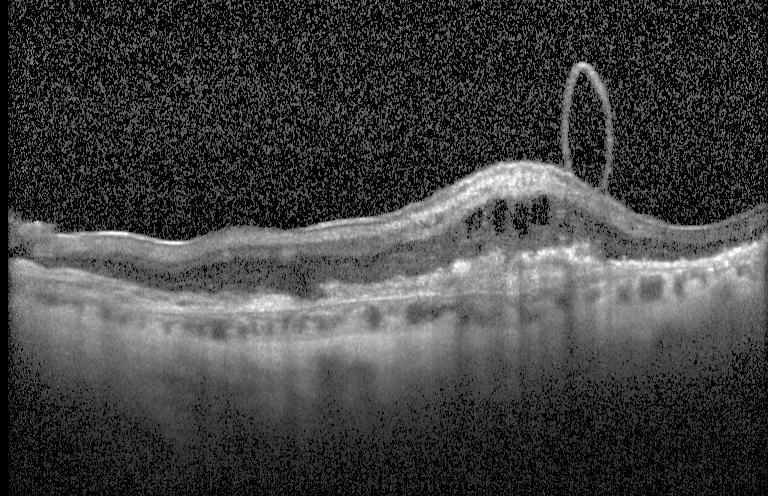

OCT B-scan showing a choroidal neovascular membrane.